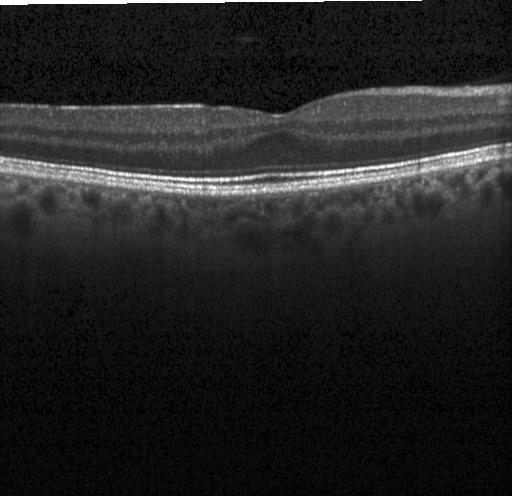 Instrument: Heidelberg Spectralis. Spectral-domain OCT. Optical coherence tomography scan. Centered on the fovea — No choroidal neovascularization, diabetic macular edema, or drusen.